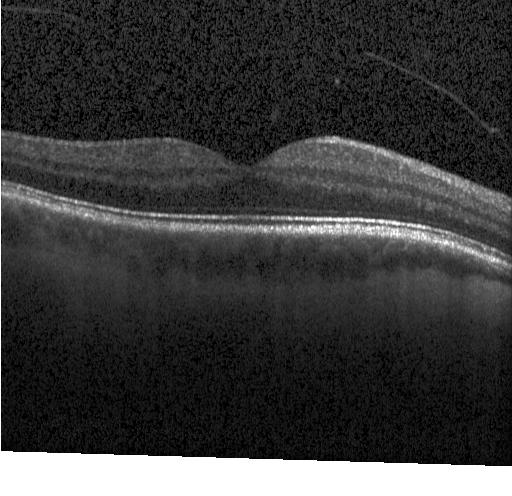 Heidelberg Spectralis OCT system · retinal OCT B-scan.
Finding: no evidence of CNV, DME, or drusen.